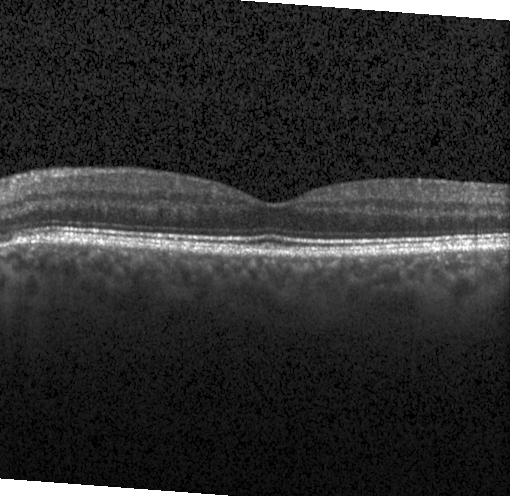

Spectral-domain OCT; fovea-centered; OCT line scan.
Finding: no evidence of CNV, DME, or drusen.